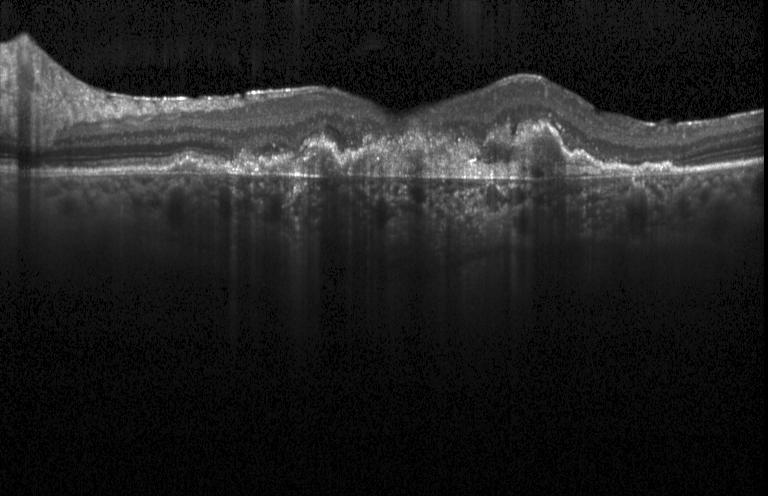
OCT line scan; centered on the fovea.
Diagnosis: choroidal neovascularization (CNV).